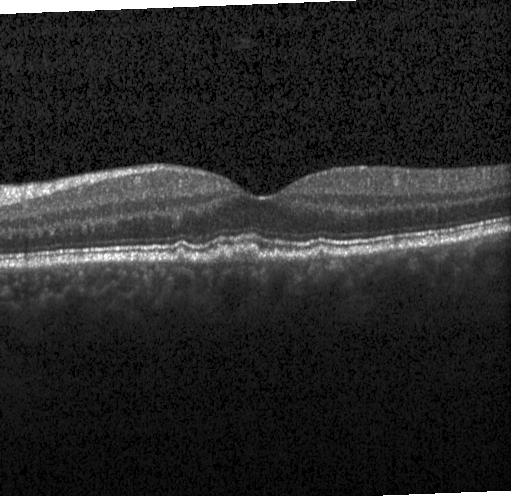
Macular scan. Heidelberg Spectralis OCT system. Optical coherence tomography B-scan. Spectral-domain OCT. Assessment: sub-RPE drusenoid deposits.